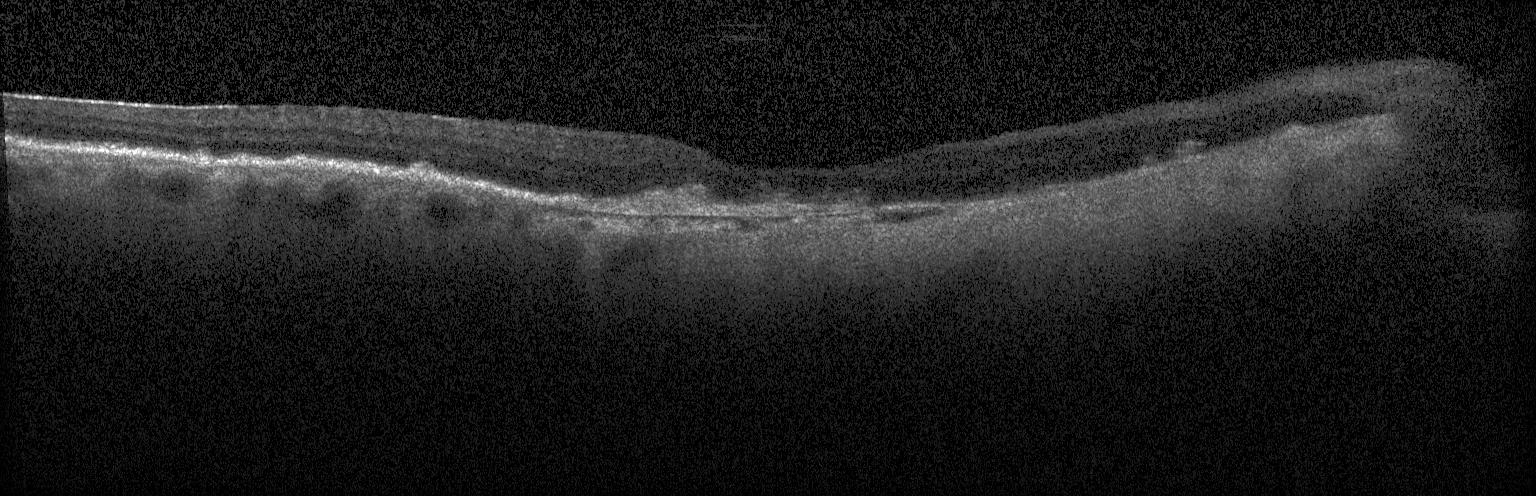

Impression: a choroidal neovascular membrane.